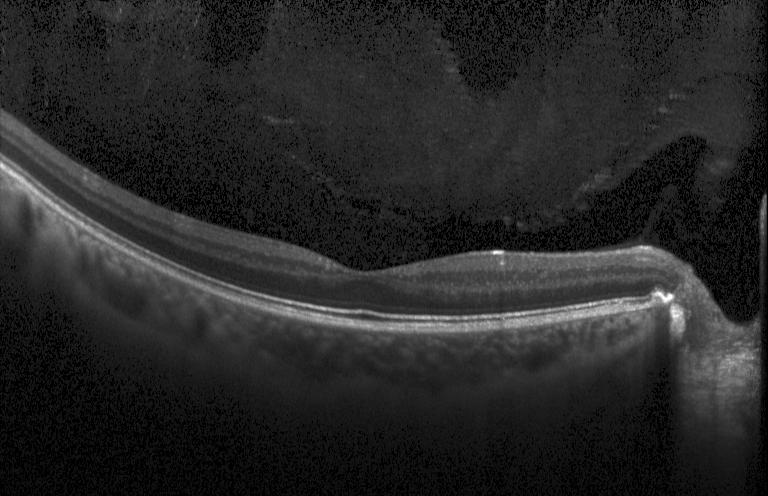
Acquired on a Heidelberg Spectralis · OCT B-scan. Diagnosis: no evidence of CNV, DME, or drusen.